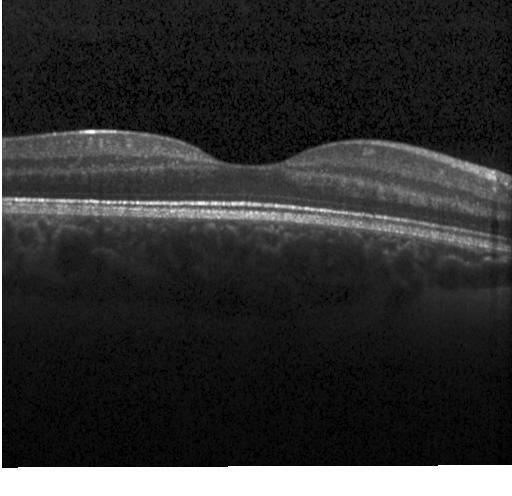

OCT finding: neither choroidal neovascularization, diabetic macular edema, nor drusen.